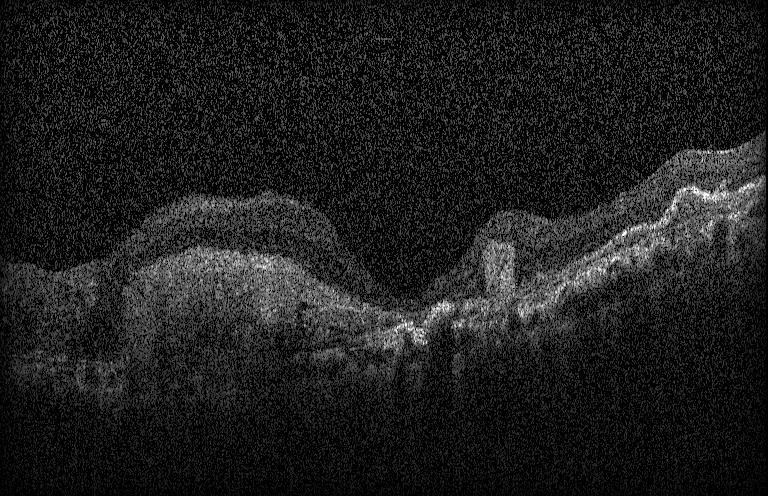

Acquired on a Heidelberg Spectralis; optical coherence tomography B-scan; centered on the fovea; spectral-domain optical coherence tomography — Diagnosis: a choroidal neovascular membrane.